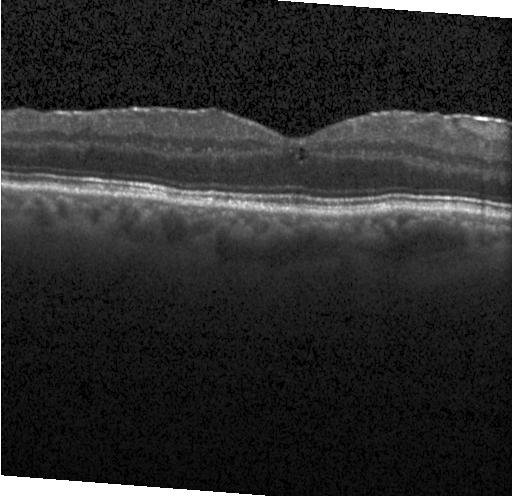 Through the macula; retinal OCT B-scan; acquired on a Heidelberg Spectralis; SD-OCT — Assessment: DME.